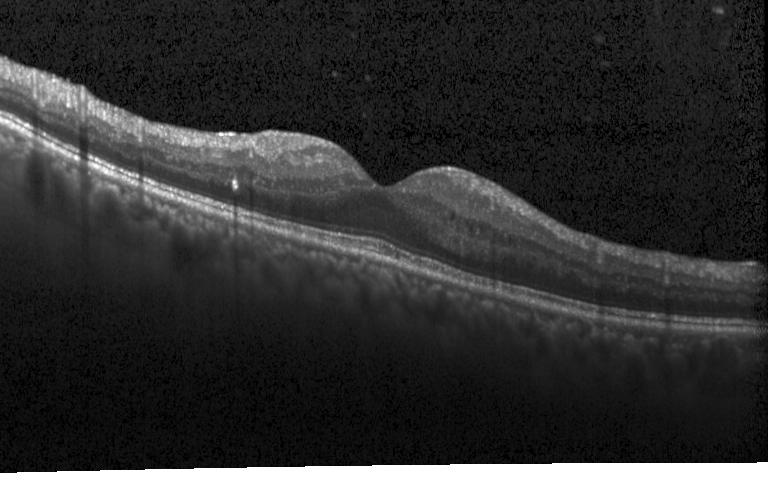
Diagnosis: no evidence of choroidal neovascularization, diabetic macular edema, or drusen.